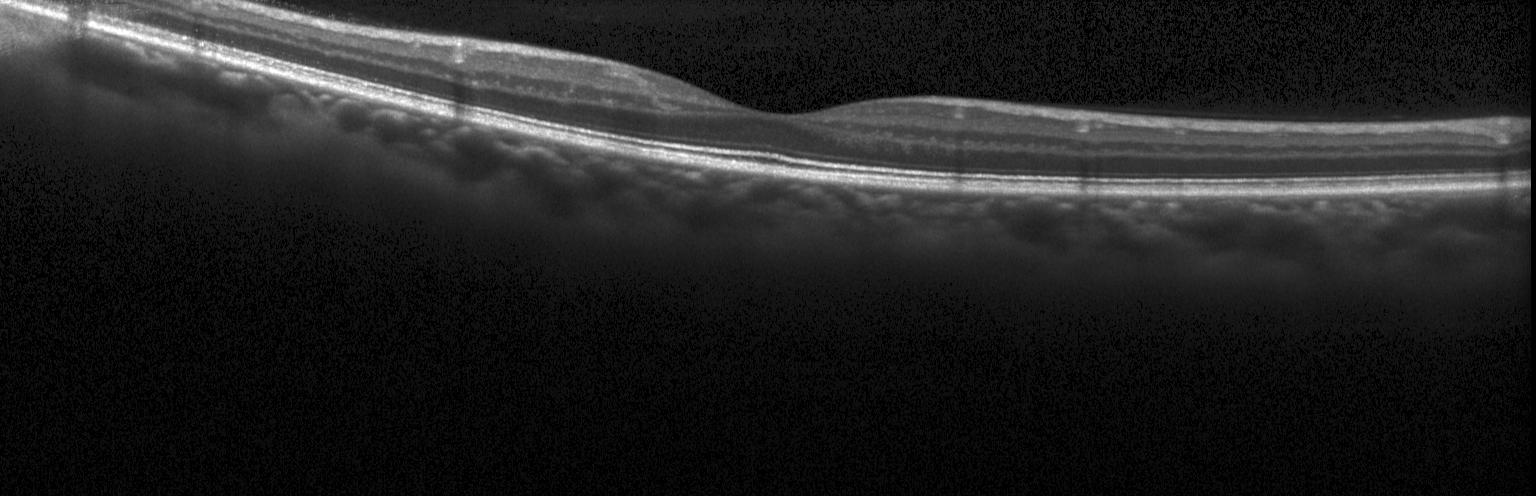 Centered on the fovea. Instrument: Heidelberg Spectralis. Retinal OCT B-scan. Finding: no evidence of choroidal neovascularization, diabetic macular edema, or drusen.